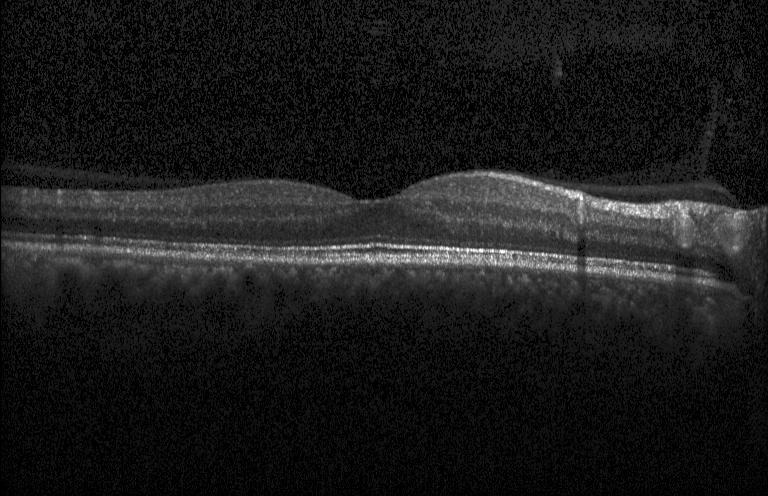 Dx: neither choroidal neovascularization, diabetic macular edema, nor drusen.